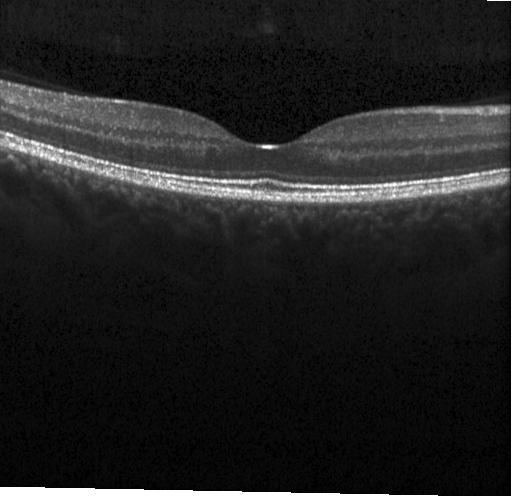

Spectral-domain OCT. Optical coherence tomography scan.
Neither choroidal neovascularization, diabetic macular edema, nor drusen.